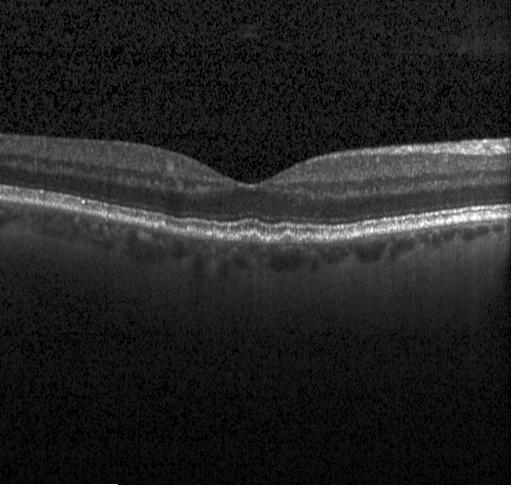 Spectral-domain OCT · Heidelberg Spectralis · optical coherence tomography scan — Diagnosis: sub-RPE drusenoid deposits.